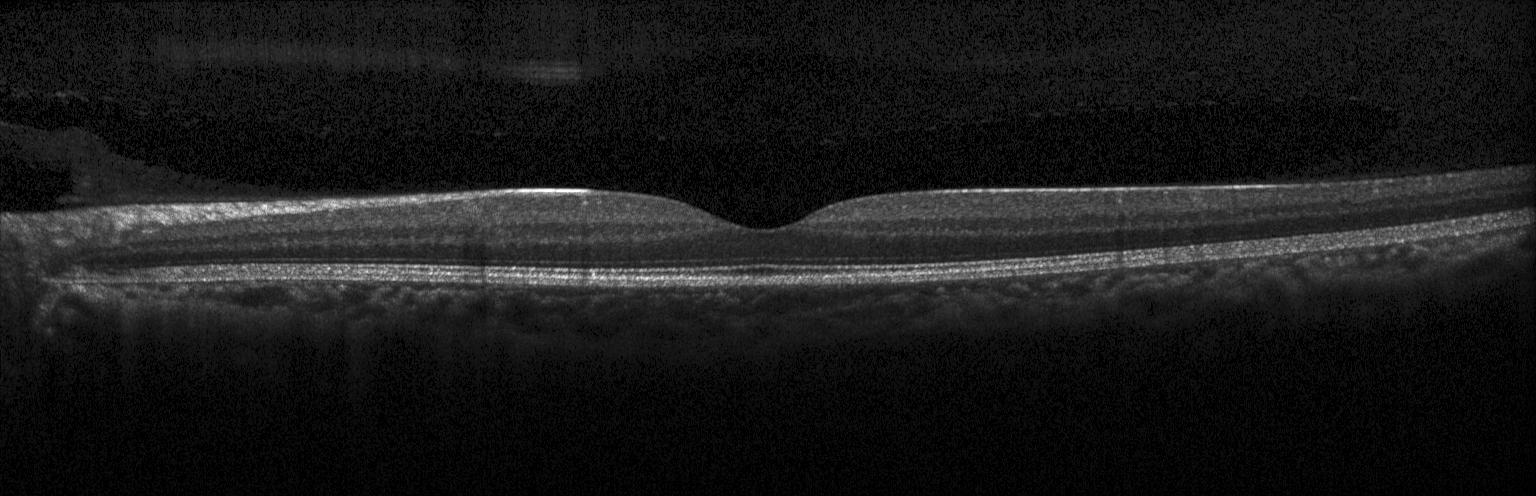

Retinal OCT cross-section showing no choroidal neovascularization, no diabetic macular edema, and no drusen.